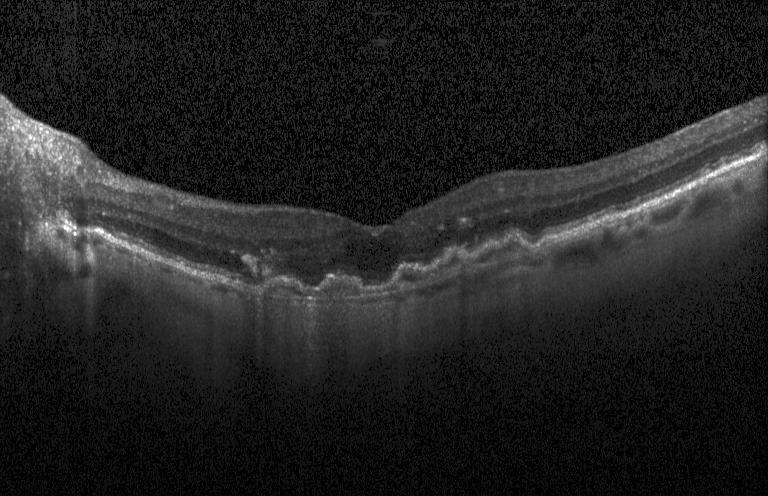
Diagnosis: choroidal neovascularization (CNV).